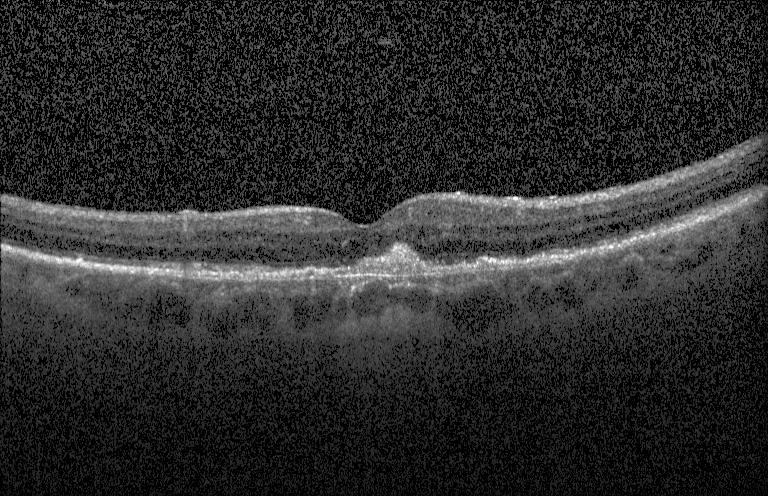 Optical coherence tomography B-scan.
Assessment: choroidal neovascularization (CNV).